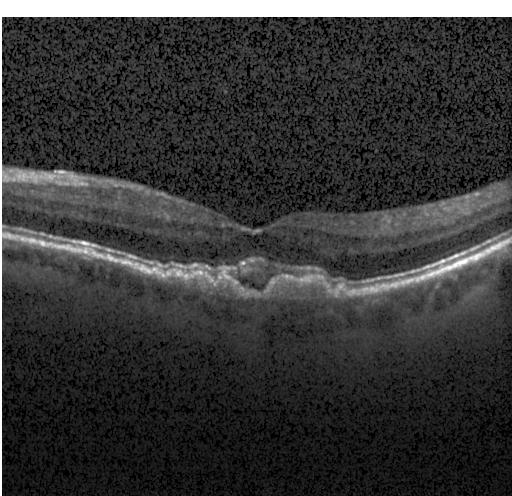 OCT line scan.
The scan shows drusen.